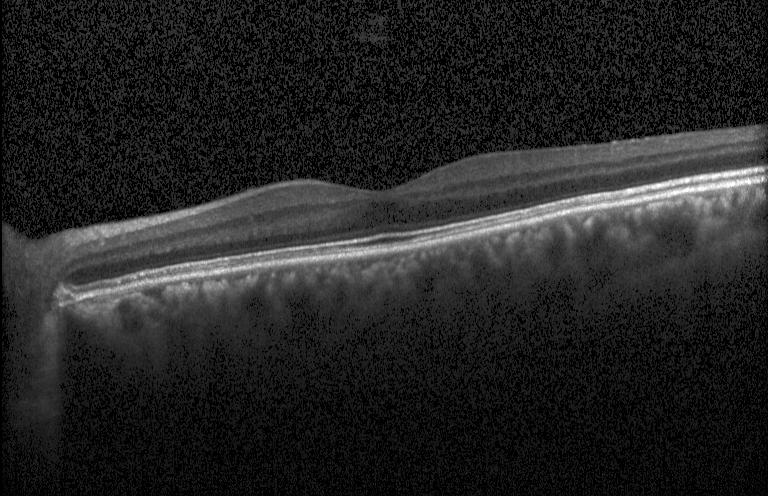 Dx: neither choroidal neovascularization, diabetic macular edema, nor drusen.